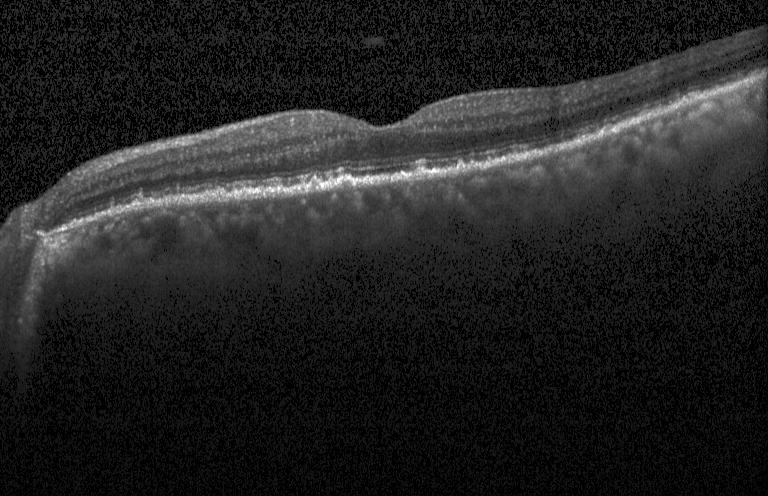
Heidelberg Spectralis OCT system. SD-OCT. OCT line scan. Through the macula. The scan shows multiple drusen.